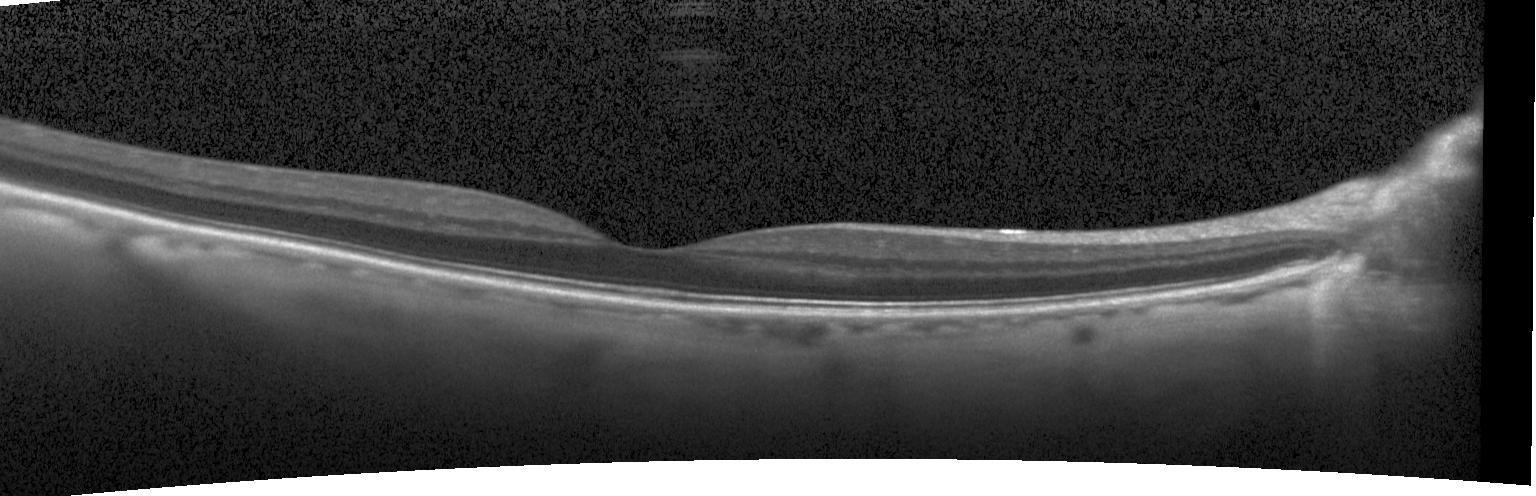

Macular scan. Optical coherence tomography B-scan — Finding: no choroidal neovascularization, diabetic macular edema, or drusen.